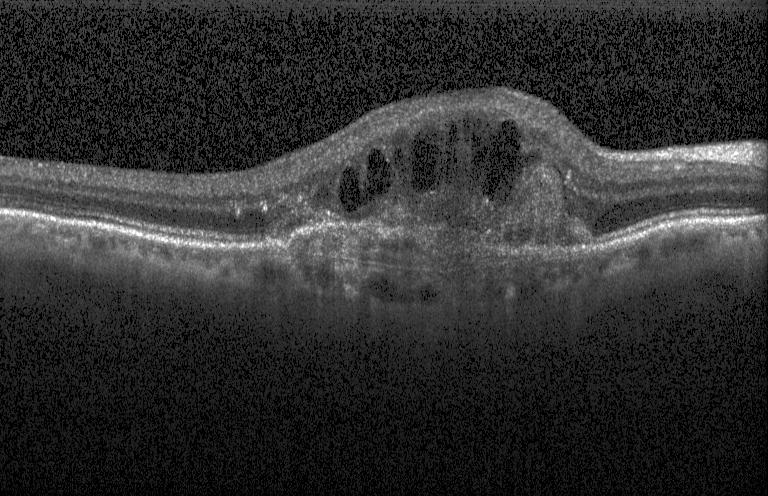

Spectral-domain OCT, centered on the fovea, optical coherence tomography B-scan. OCT finding: a choroidal neovascular membrane.